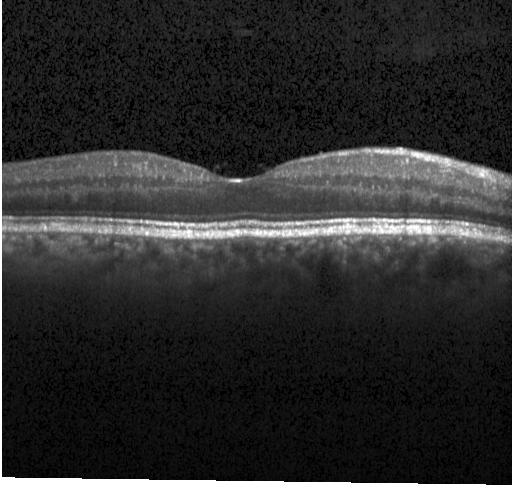

Spectral-domain optical coherence tomography · optical coherence tomography B-scan.
The scan shows neither choroidal neovascularization, diabetic macular edema, nor drusen.